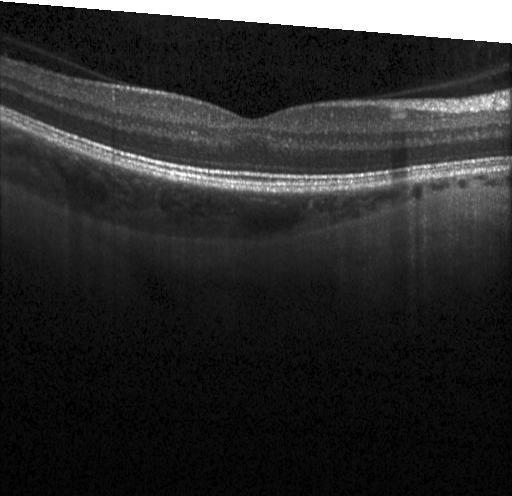

OCT B-scan showing no CNV, DME, or drusen.